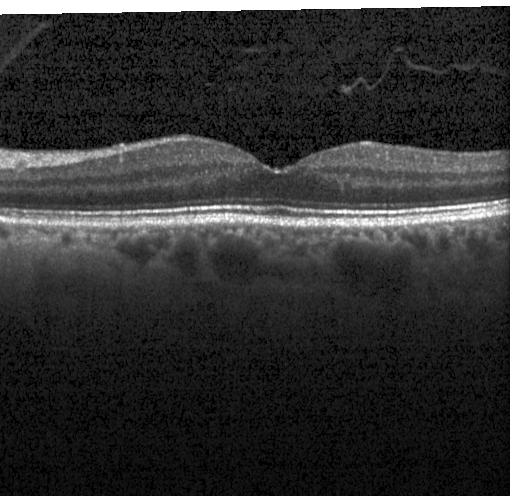 Instrument: Heidelberg Spectralis. OCT B-scan. Spectral-domain OCT — Impression: no evidence of choroidal neovascularization, diabetic macular edema, or drusen.